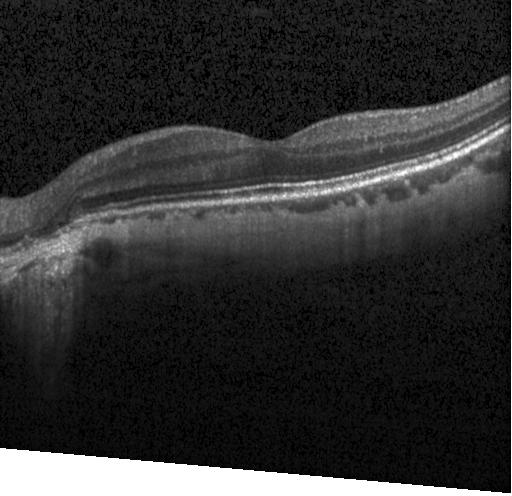 Macular OCT: no CNV, no DME, and no drusen.